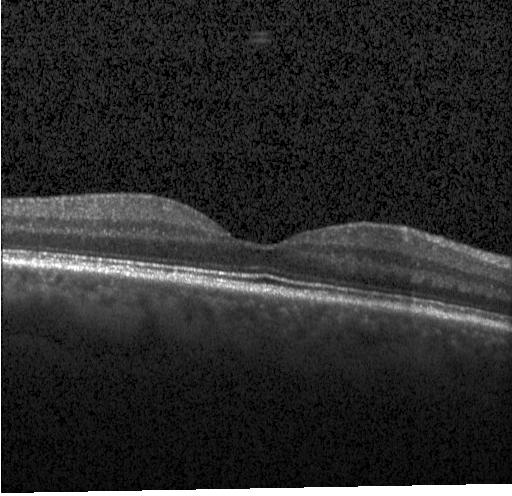 OCT B-scan.
Assessment: neither choroidal neovascularization, diabetic macular edema, nor drusen.